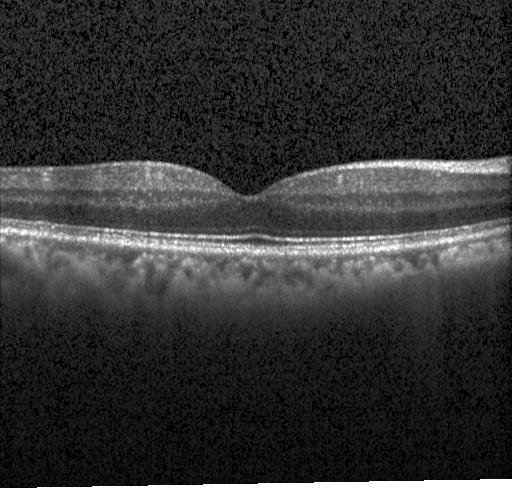 Optical coherence tomography scan · horizontal scan through the fovea · acquired on a Heidelberg Spectralis
No choroidal neovascularization, no diabetic macular edema, and no drusen.